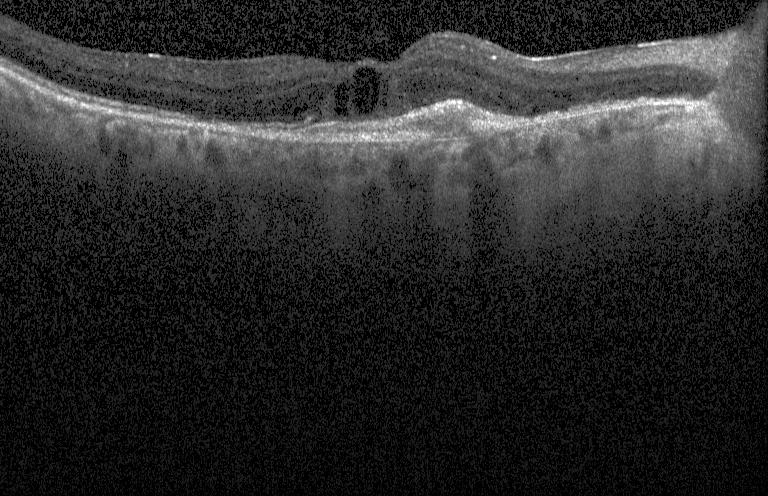
Dx: CNV.